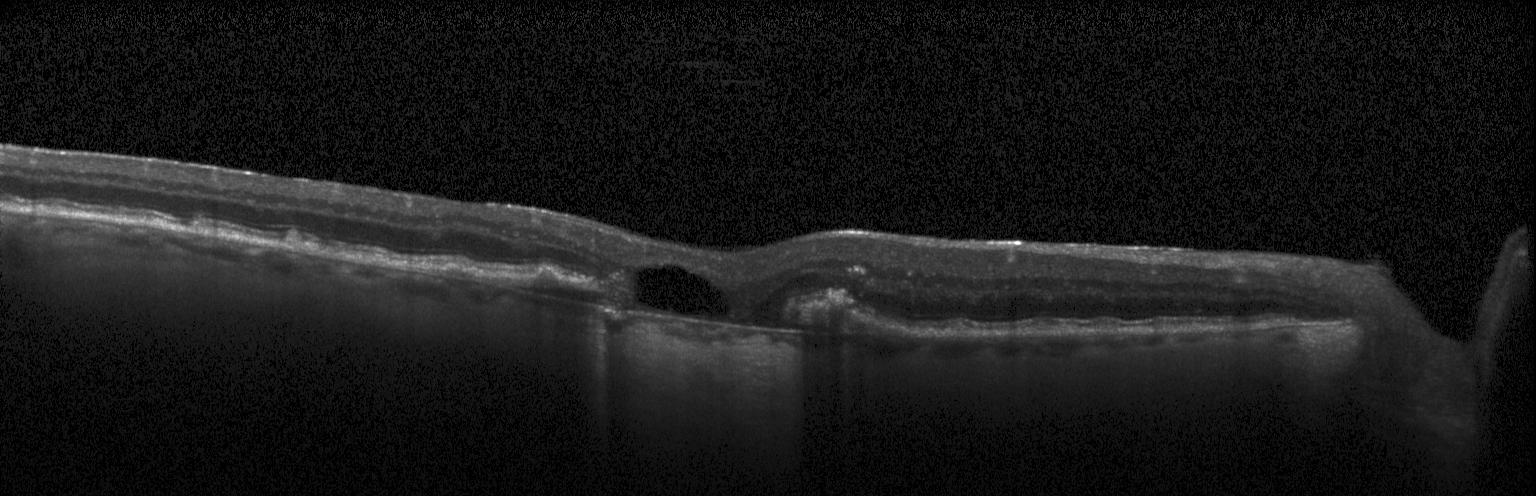 Macular OCT demonstrating choroidal neovascularization (CNV).